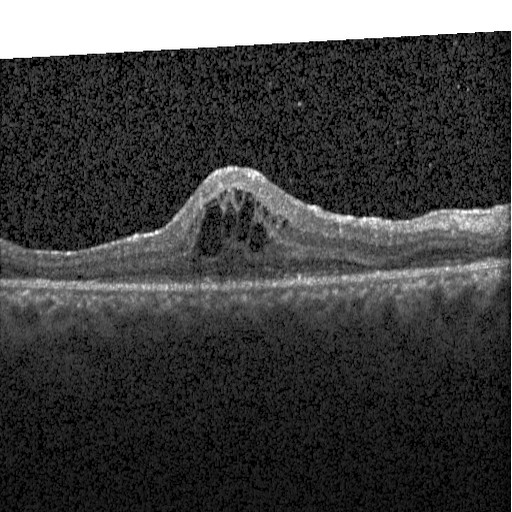

Impression: DME.